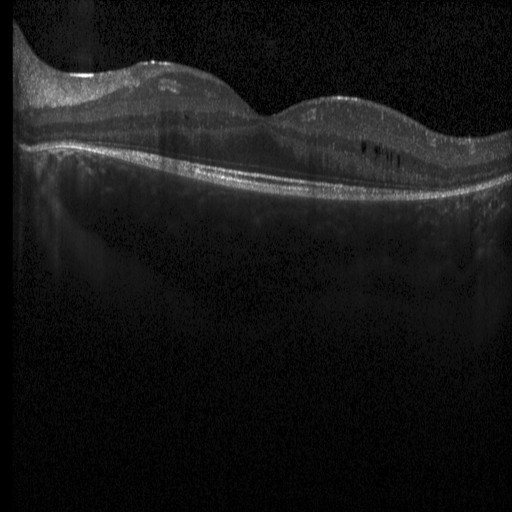
OCT finding: DME.